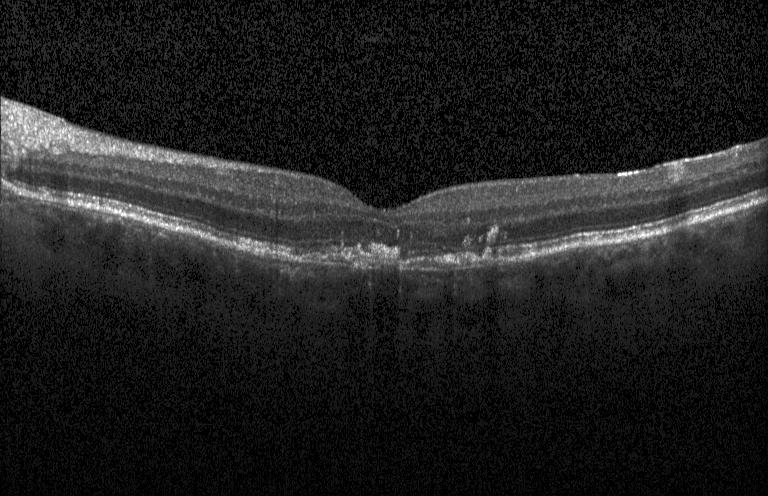

Spectral-domain OCT; acquired on a Heidelberg Spectralis; OCT line scan; centered on the fovea. Macular OCT: choroidal neovascularization.